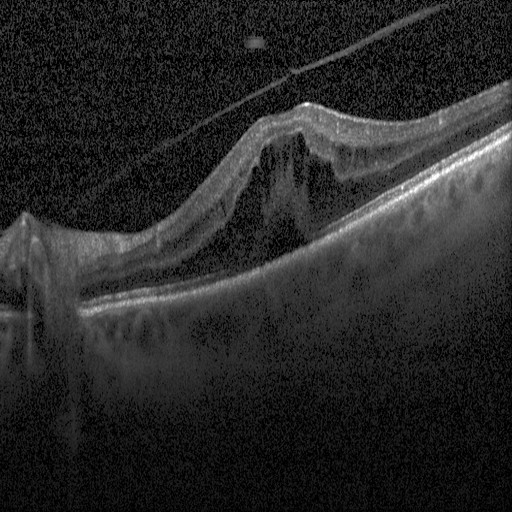 Retinal OCT cross-section; Heidelberg Spectralis. Finding: diabetic macular edema.